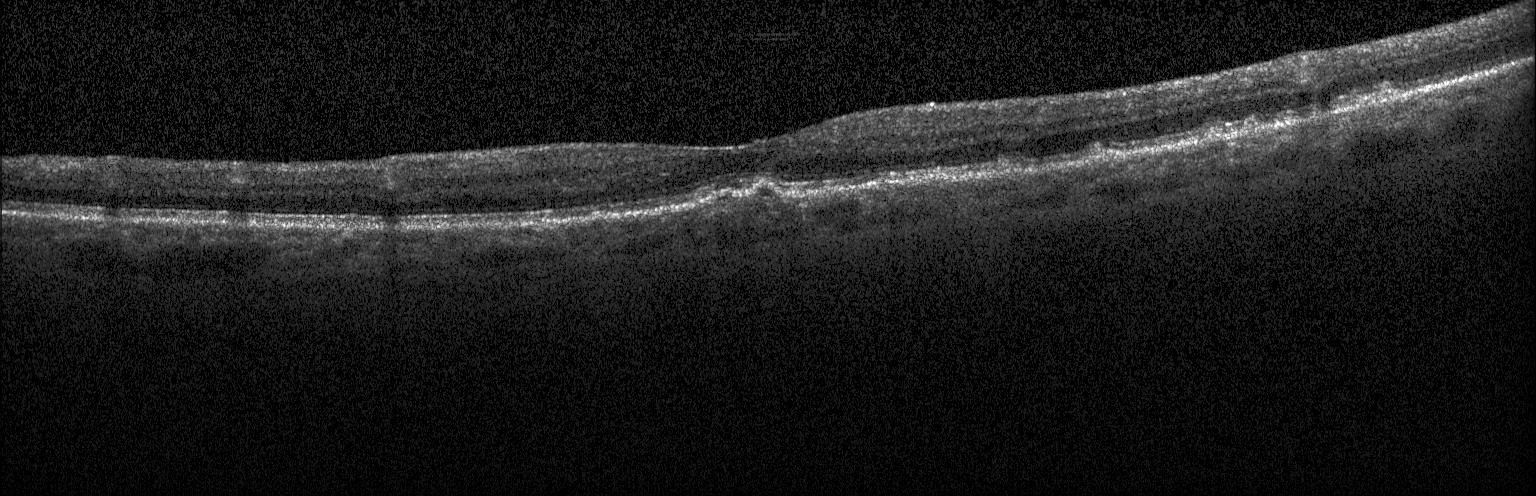

OCT line scan · fovea-centered · SD-OCT · instrument: Heidelberg Spectralis
Impression: drusen.